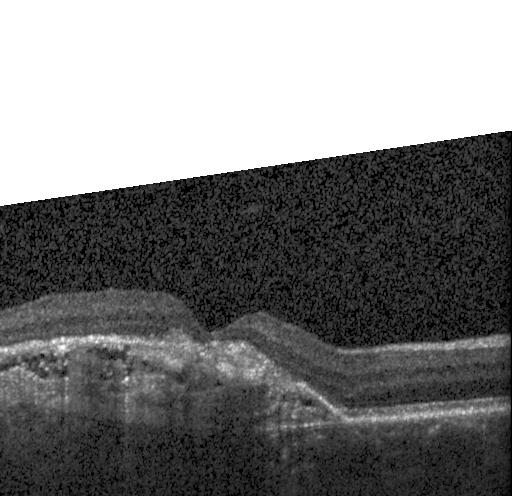
Spectral-domain optical coherence tomography; through the macula; retinal OCT cross-section; acquired on a Heidelberg Spectralis. Impression: choroidal neovascularization (CNV).